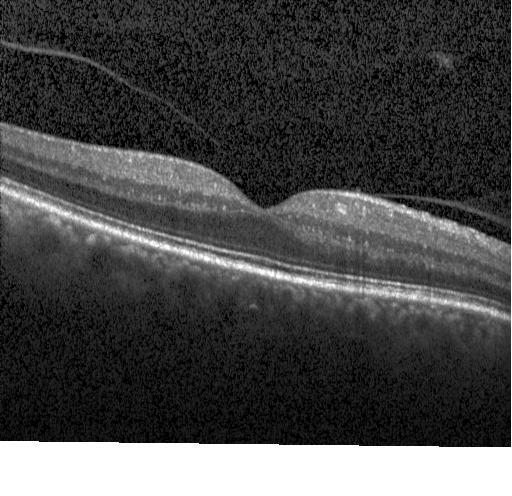 OCT line scan · acquired on a Heidelberg Spectralis.
Finding: no evidence of choroidal neovascularization, diabetic macular edema, or drusen.